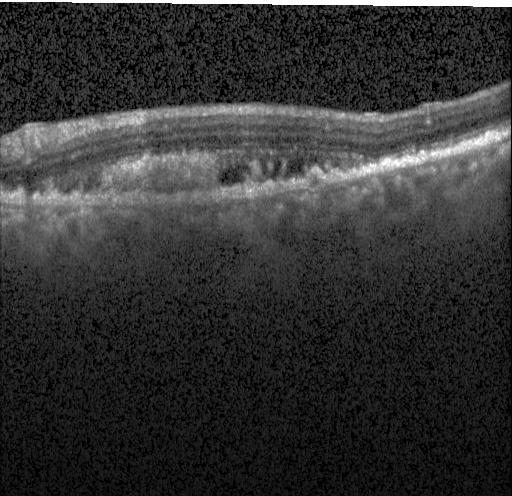
Optical coherence tomography scan.
Assessment: a choroidal neovascular membrane.